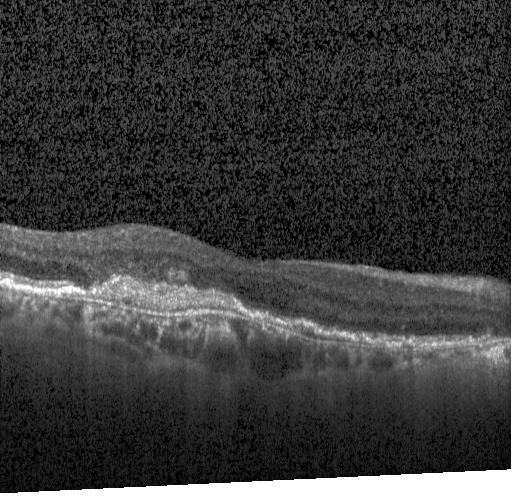

Optical coherence tomography scan
Macular OCT: choroidal neovascularization.